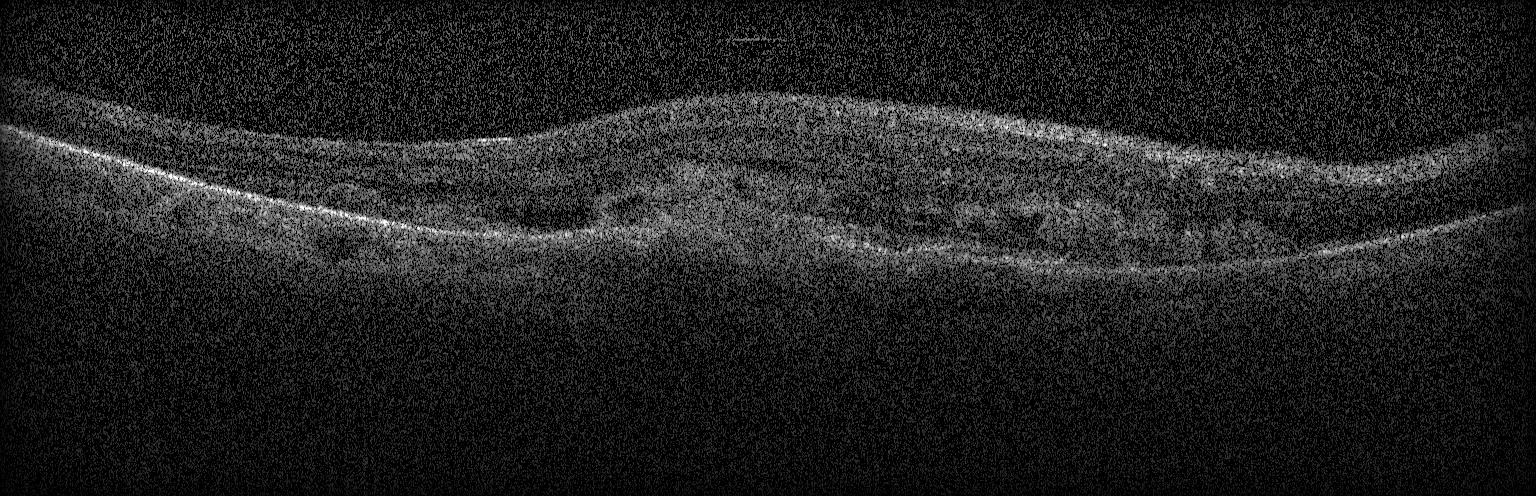 Optical coherence tomography scan. Macular OCT: choroidal neovascularization (CNV).